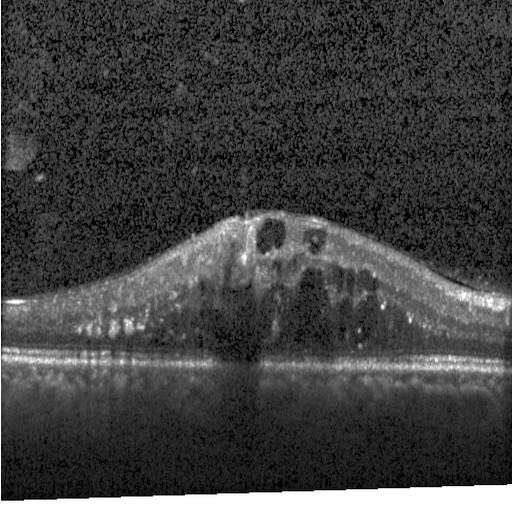 OCT line scan.
DME.